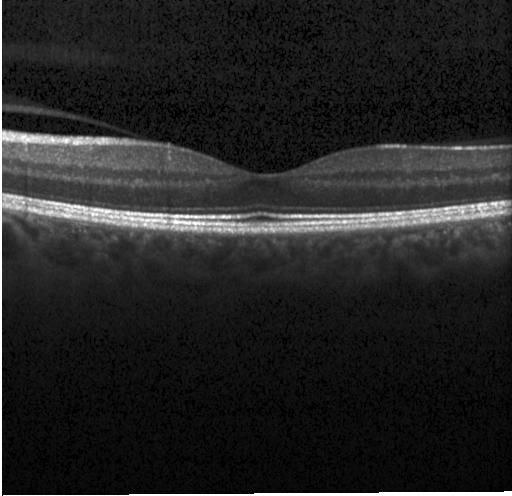

Acquired on a Heidelberg Spectralis, centered on the fovea, SD-OCT, optical coherence tomography B-scan — Finding: no choroidal neovascularization, no diabetic macular edema, and no drusen.